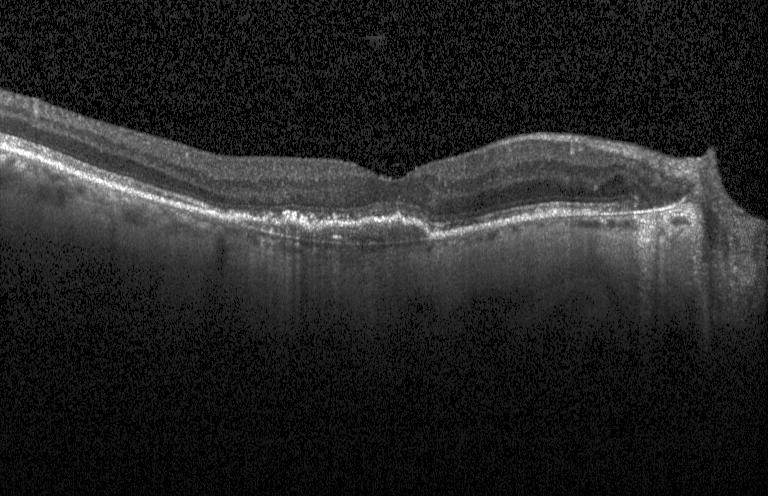 Spectral-domain optical coherence tomography; optical coherence tomography scan.
OCT finding: choroidal neovascularization.